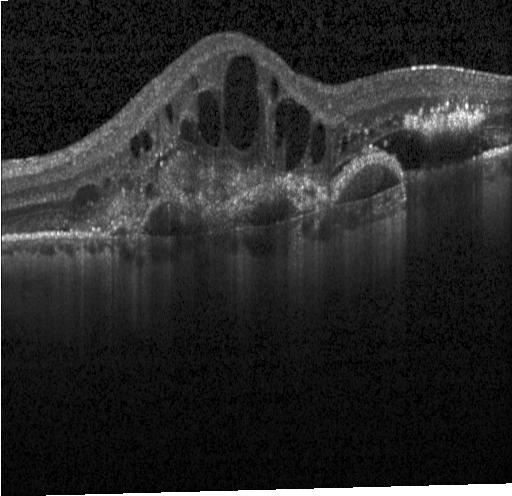

Macular scan, instrument: Heidelberg Spectralis, retinal OCT cross-section, spectral-domain optical coherence tomography — Dx: choroidal neovascularization.